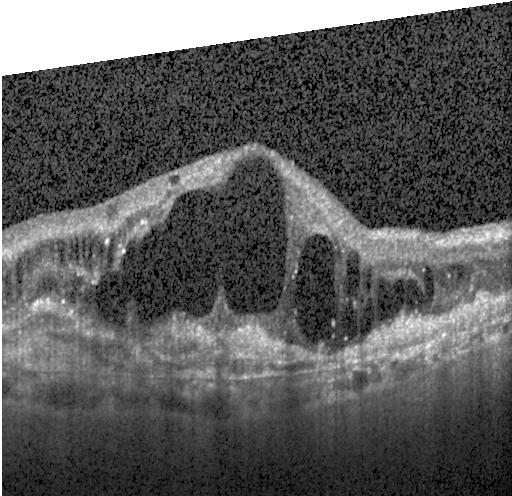

OCT B-scan. Spectral-domain optical coherence tomography. Heidelberg Spectralis OCT system
Diagnosis: choroidal neovascularization (CNV).